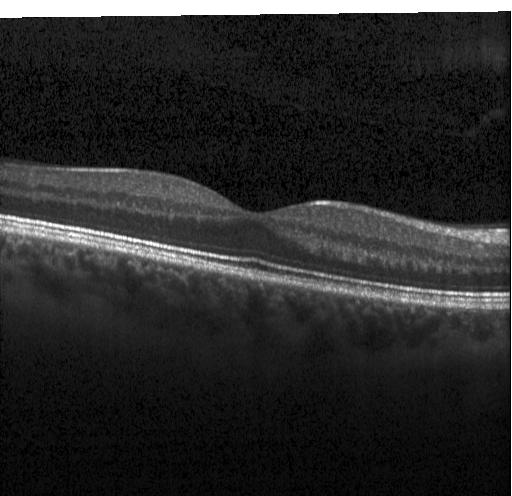

Diagnosis: no choroidal neovascularization, no diabetic macular edema, and no drusen.